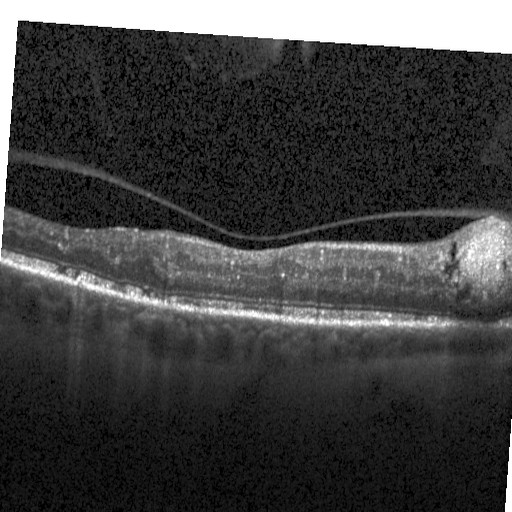

OCT line scan, fovea-centered, Heidelberg Spectralis OCT system, SD-OCT.
Impression: diabetic macular edema (DME).